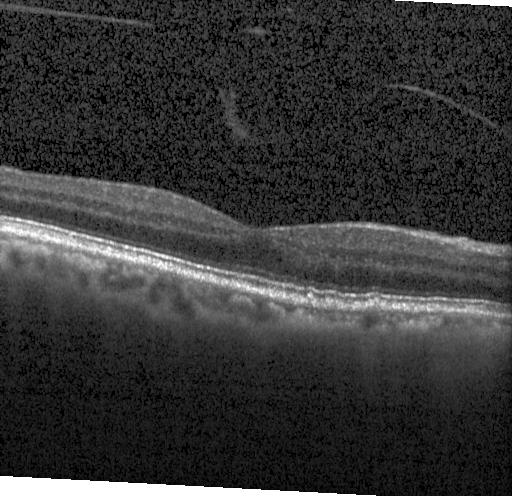 Spectral-domain OCT, optical coherence tomography scan, instrument: Heidelberg Spectralis.
Assessment: drusen.